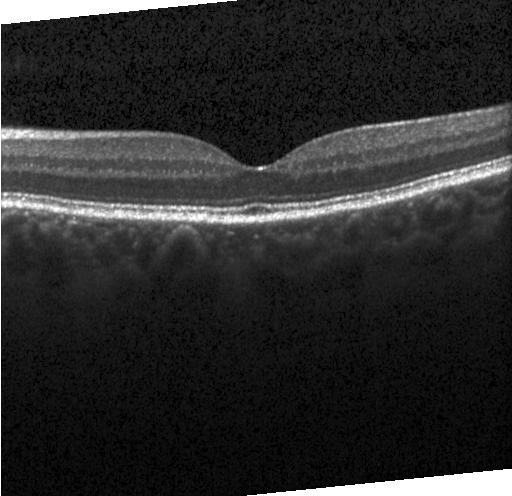

No evidence of choroidal neovascularization, diabetic macular edema, or drusen.